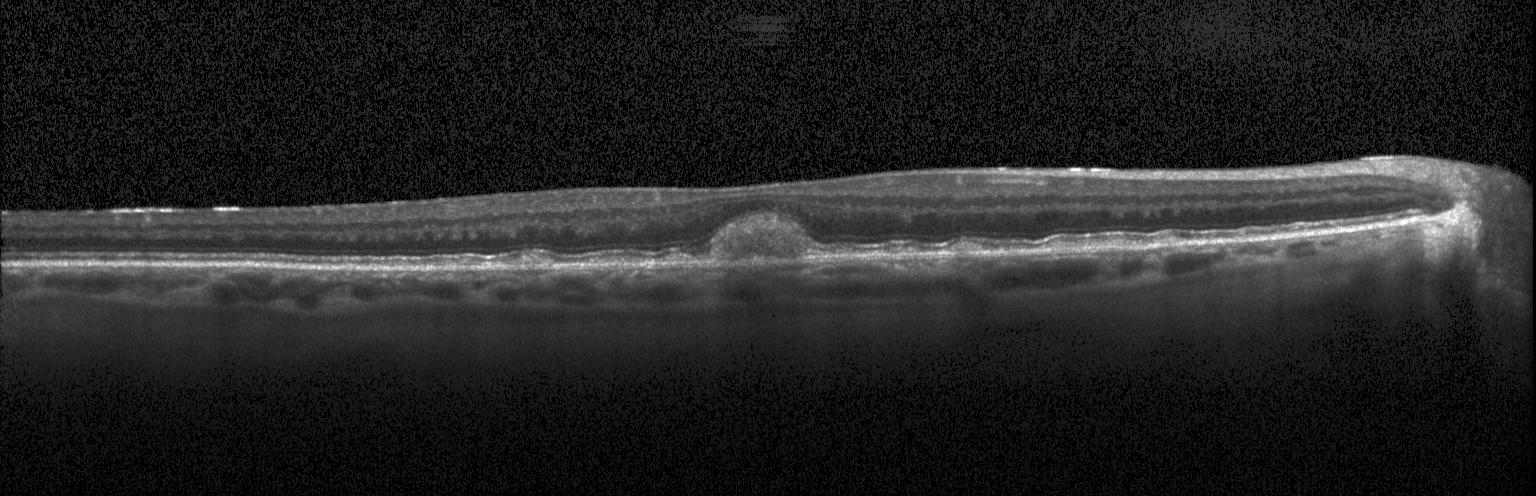

Macular OCT: CNV.